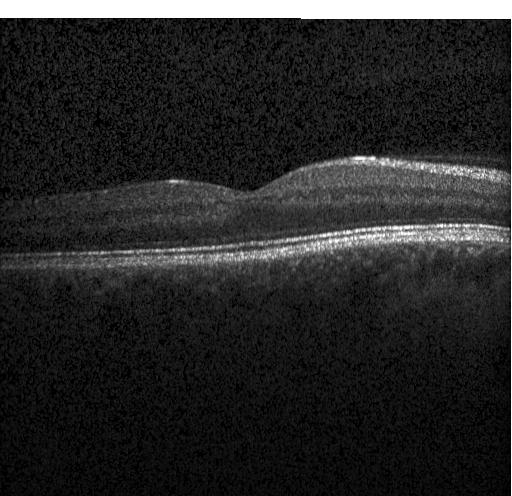
Retinal OCT B-scan — Finding: no CNV, DME, or drusen.